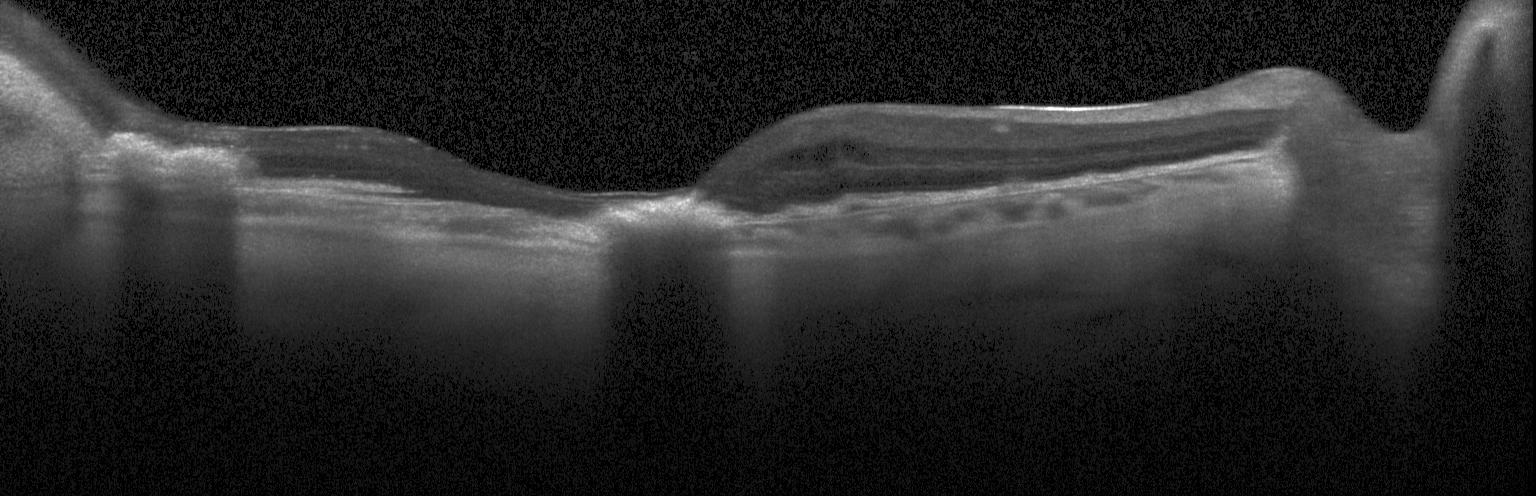
A choroidal neovascular membrane.